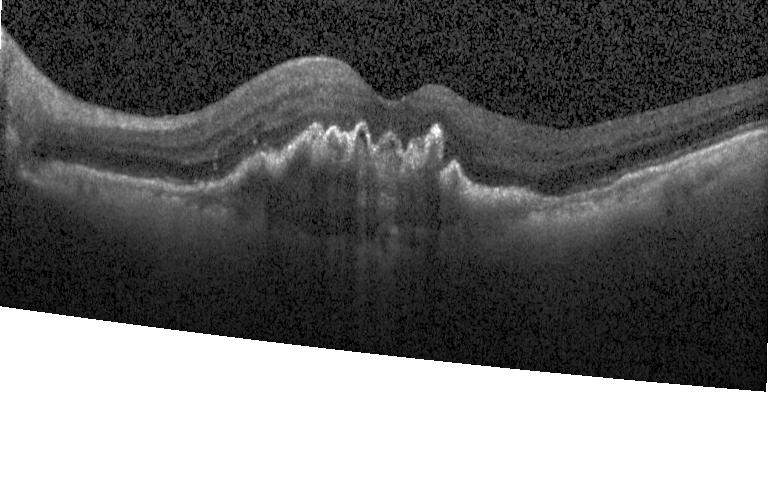 OCT line scan, horizontal scan through the fovea, Heidelberg Spectralis OCT system. Macular OCT: choroidal neovascularization.